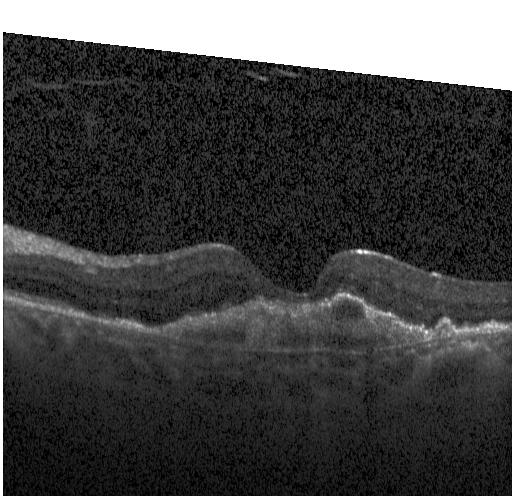 Retinal OCT cross-section. Impression: choroidal neovascularization (CNV).